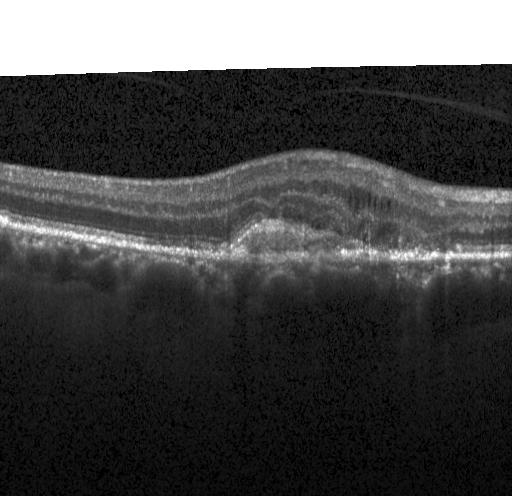
Acquired on a Heidelberg Spectralis, retinal OCT cross-section
Impression: a choroidal neovascular membrane.